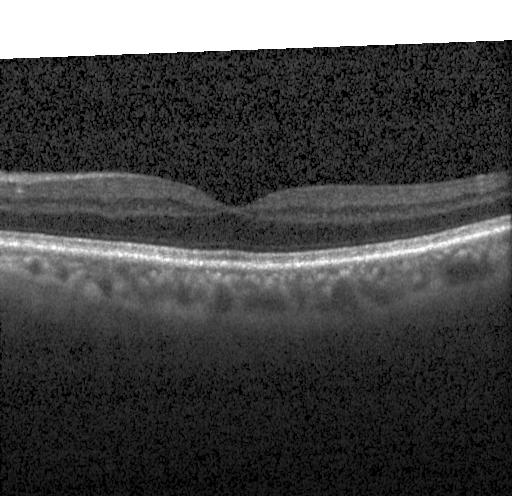 The scan shows neither choroidal neovascularization, diabetic macular edema, nor drusen.